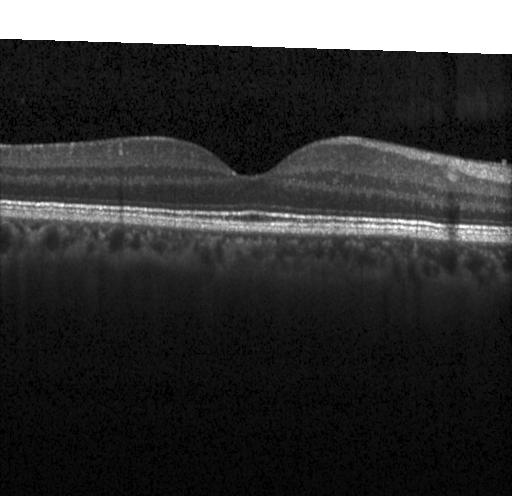

Instrument: Heidelberg Spectralis, through the macula, spectral-domain OCT, retinal OCT B-scan — Finding: no choroidal neovascularization, no diabetic macular edema, and no drusen.